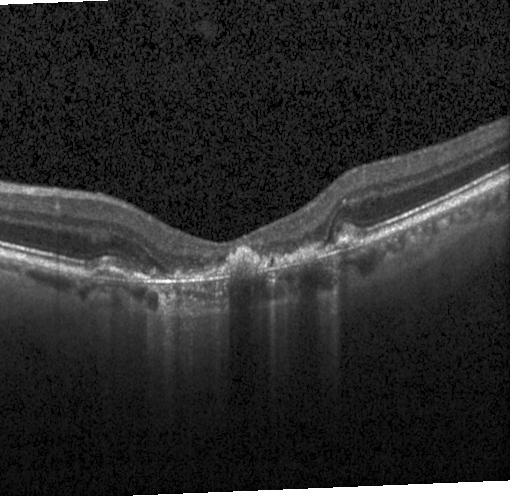

Heidelberg Spectralis OCT system, fovea-centered, retinal OCT cross-section, SD-OCT
Impression: choroidal neovascularization.